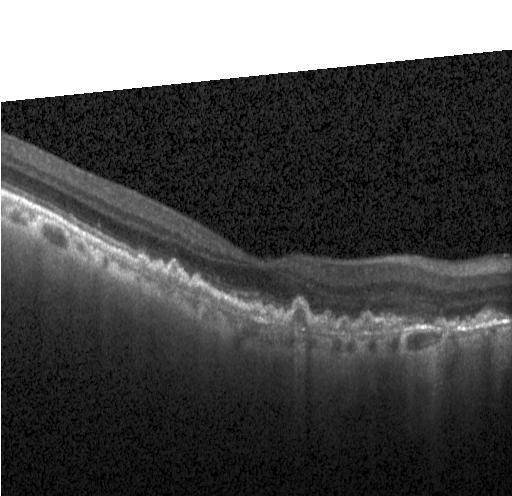 OCT B-scan. Impression: a choroidal neovascular membrane.